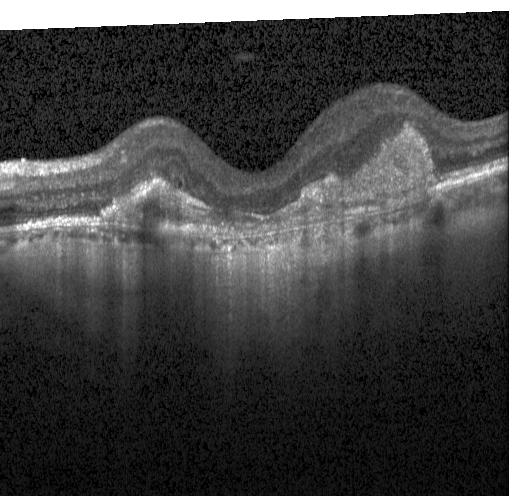 Diagnosis: choroidal neovascularization.